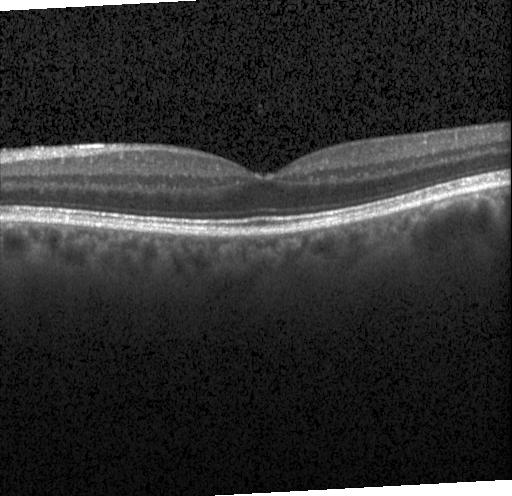 Macular OCT: no choroidal neovascularization, diabetic macular edema, or drusen.